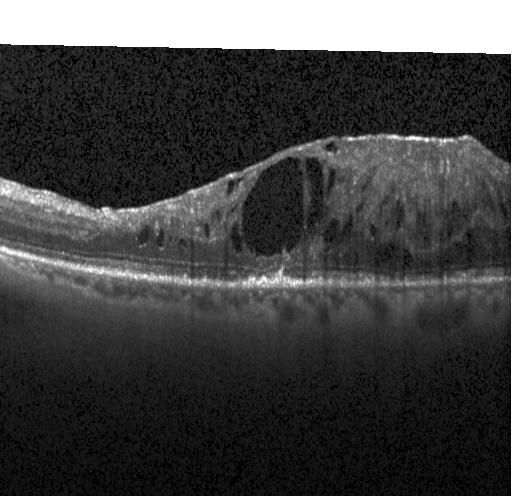

Heidelberg Spectralis · optical coherence tomography B-scan
Dx: diabetic macular edema.